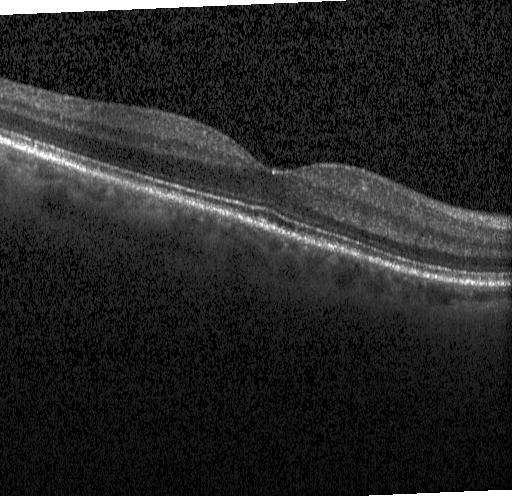
Spectral-domain OCT. Heidelberg Spectralis OCT system. Optical coherence tomography B-scan. Through the macula
Macular OCT: neither choroidal neovascularization, diabetic macular edema, nor drusen.